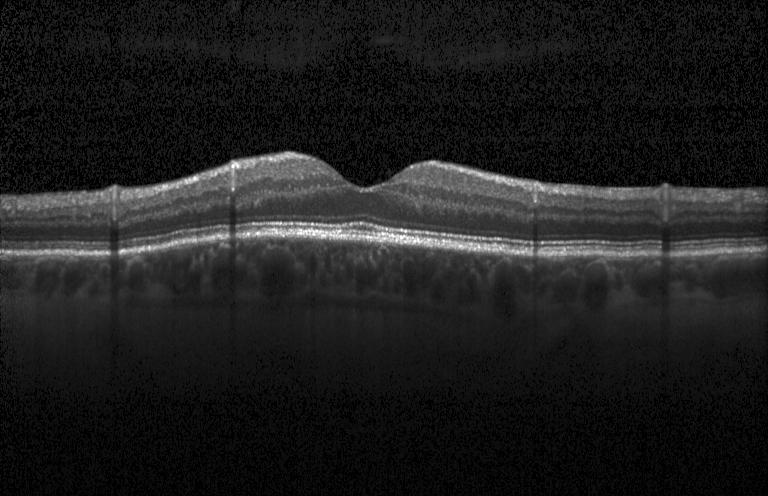

Impression: neither CNV, DME, nor drusen.